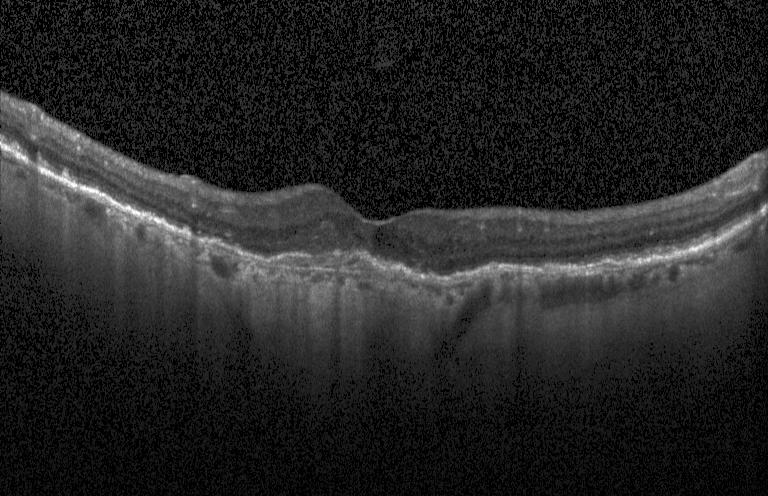 Optical coherence tomography scan, centered on the fovea, Heidelberg Spectralis — Finding: a choroidal neovascular membrane.